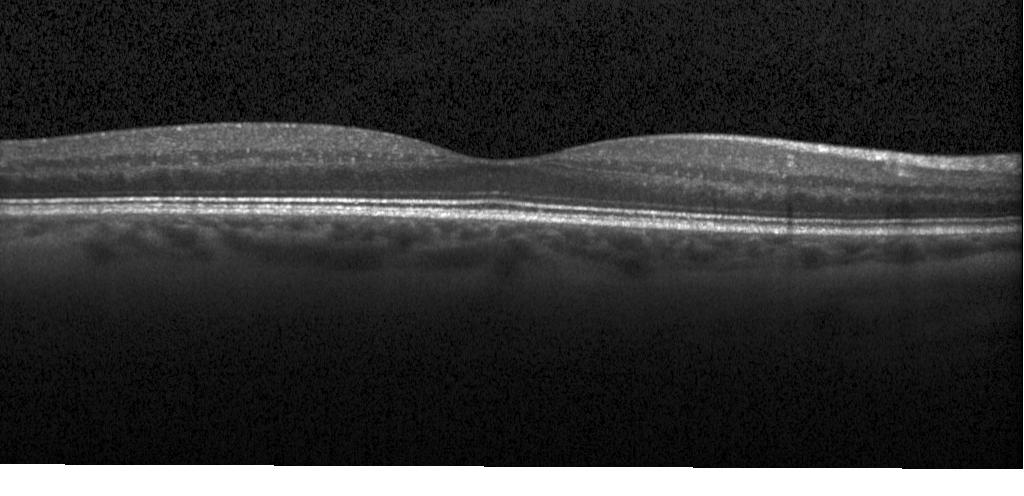
No choroidal neovascularization, no diabetic macular edema, and no drusen.